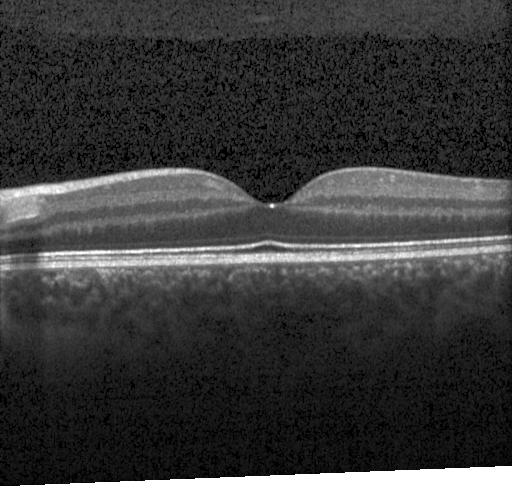 OCT line scan — Dx: no CNV, DME, or drusen.